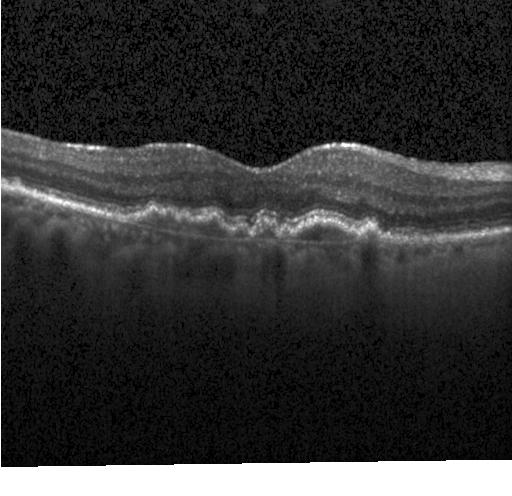

Retinal OCT B-scan.
Macular OCT: CNV.